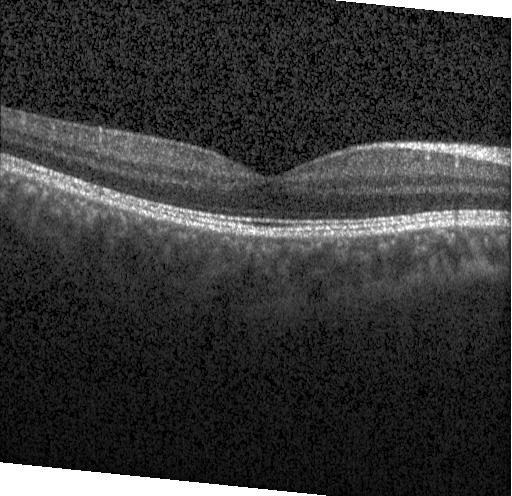

Optical coherence tomography B-scan; macular scan
Impression: no CNV, DME, or drusen.